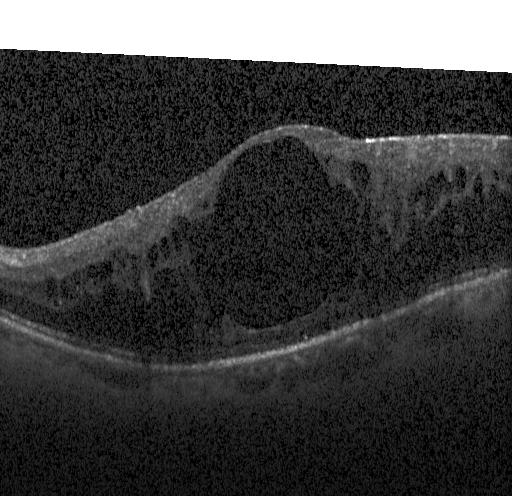
Instrument: Heidelberg Spectralis, OCT line scan. This B-scan demonstrates diabetic macular edema (DME).